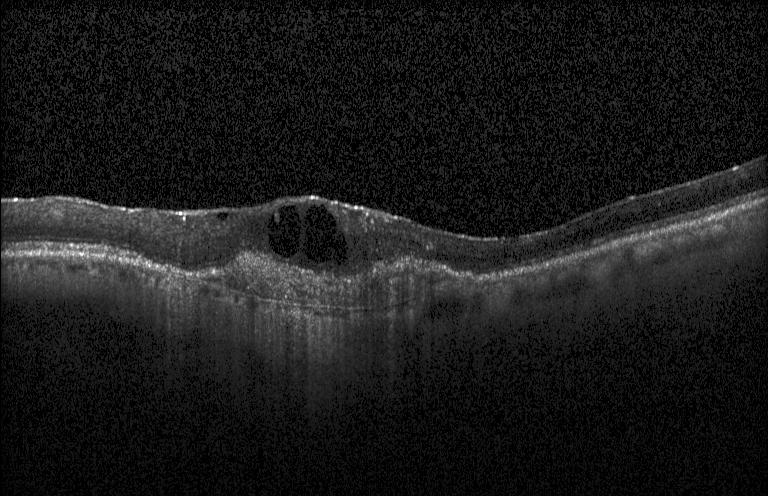 Optical coherence tomography scan · spectral-domain optical coherence tomography · acquired on a Heidelberg Spectralis · through the macula — Finding: CNV.